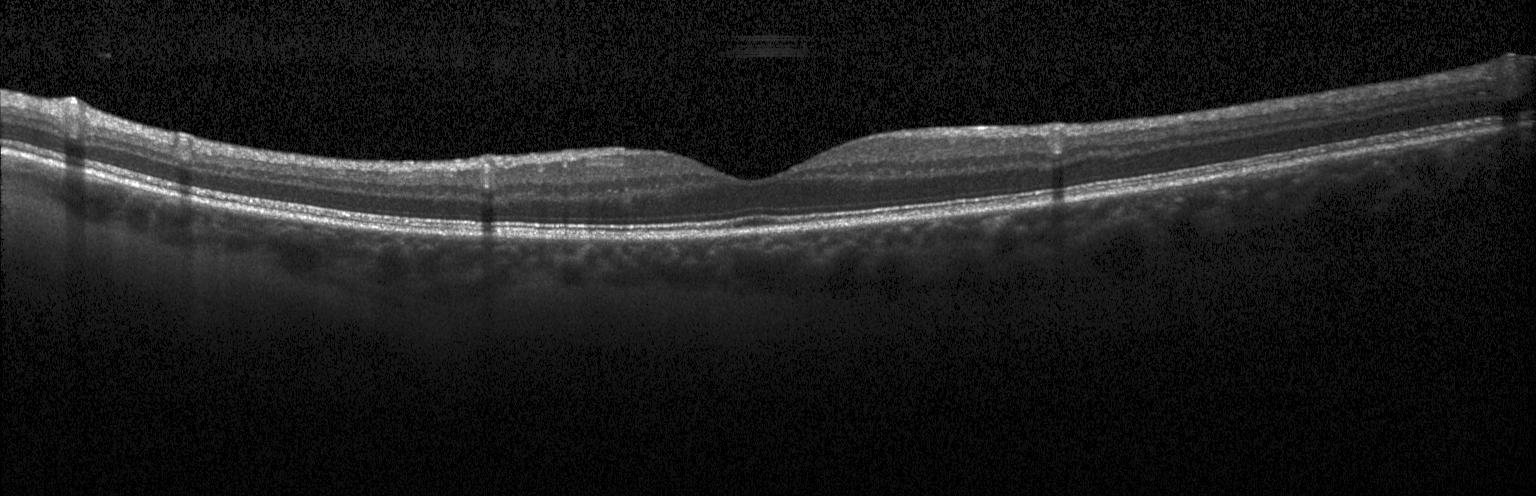
Optical coherence tomography scan · Heidelberg Spectralis OCT system
Impression: no choroidal neovascularization, no diabetic macular edema, and no drusen.